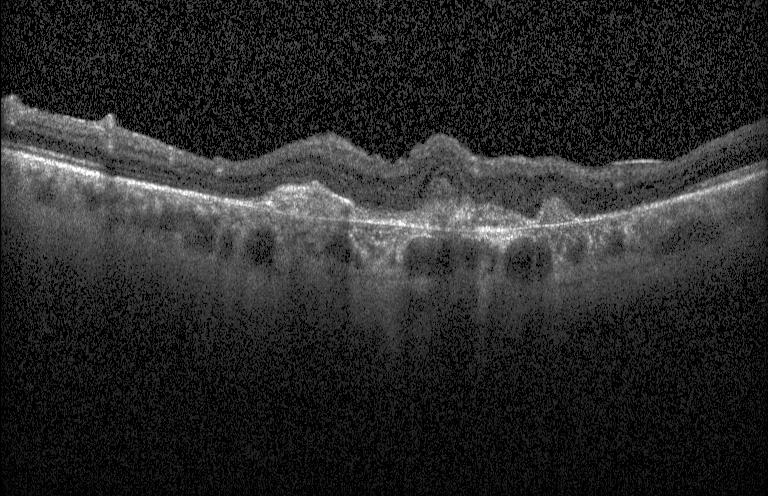 OCT B-scan, acquired on a Heidelberg Spectralis, macular scan, SD-OCT — Assessment: a choroidal neovascular membrane.